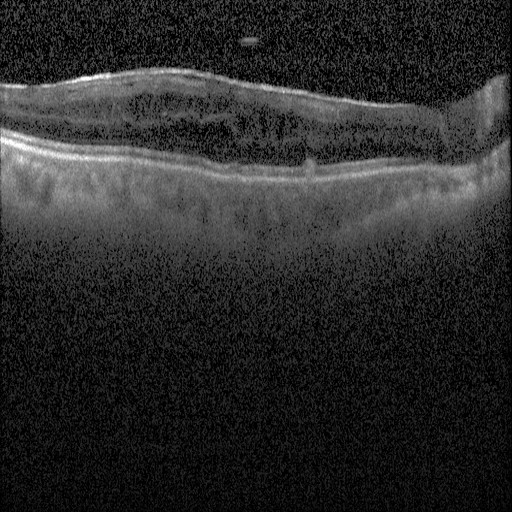 SD-OCT; OCT B-scan — This B-scan demonstrates diabetic macular edema.